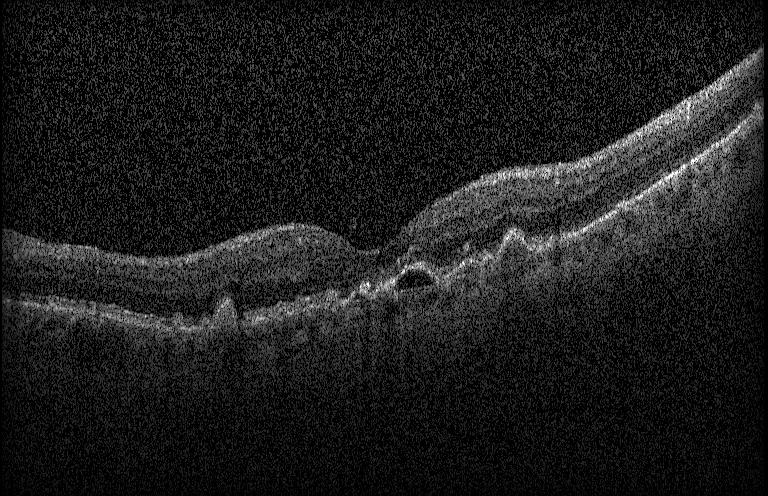 Macular OCT: a choroidal neovascular membrane.